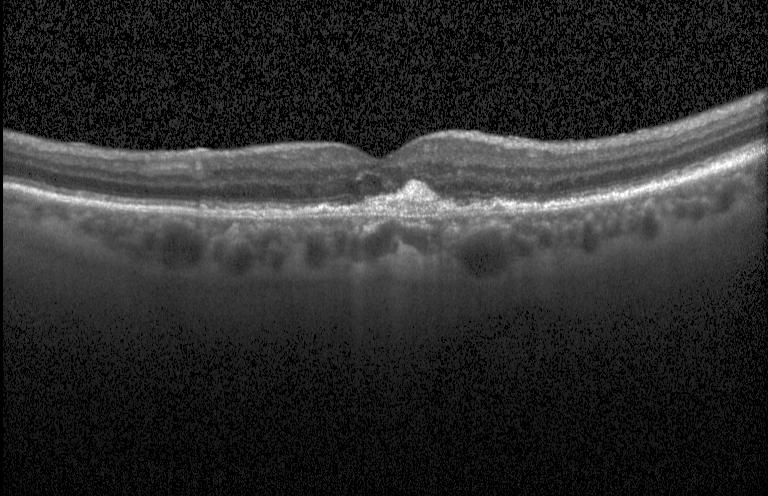

OCT B-scan
Impression: a choroidal neovascular membrane.